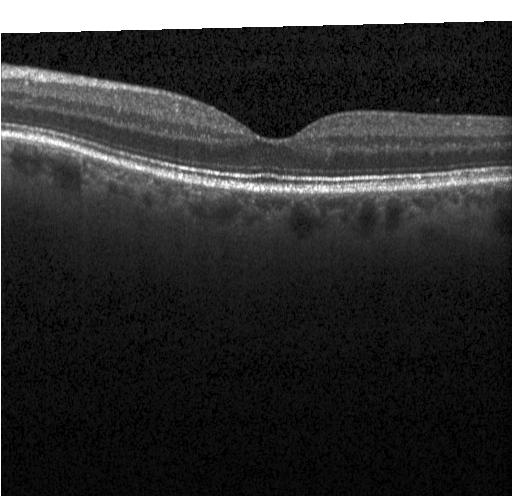
Optical coherence tomography scan; through the macula — Finding: no evidence of choroidal neovascularization, diabetic macular edema, or drusen.